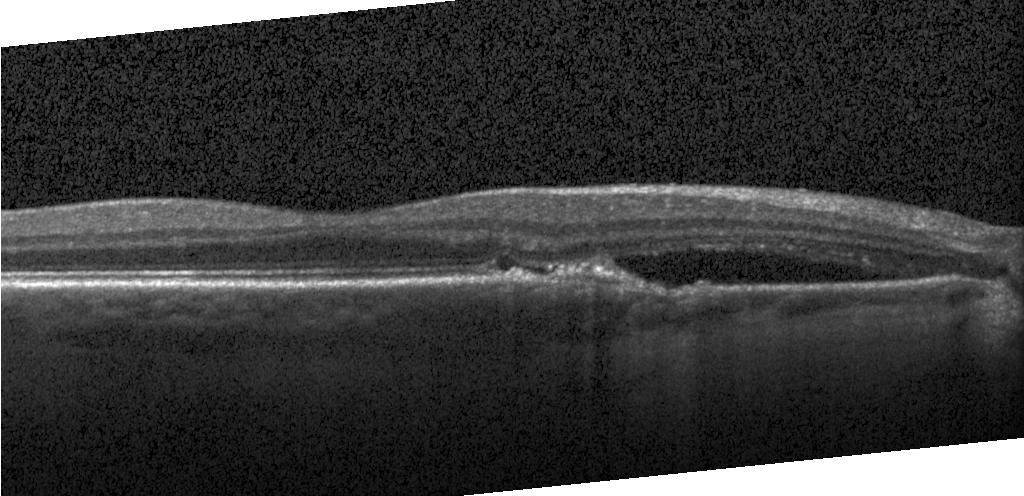 OCT B-scan showing choroidal neovascularization (CNV).